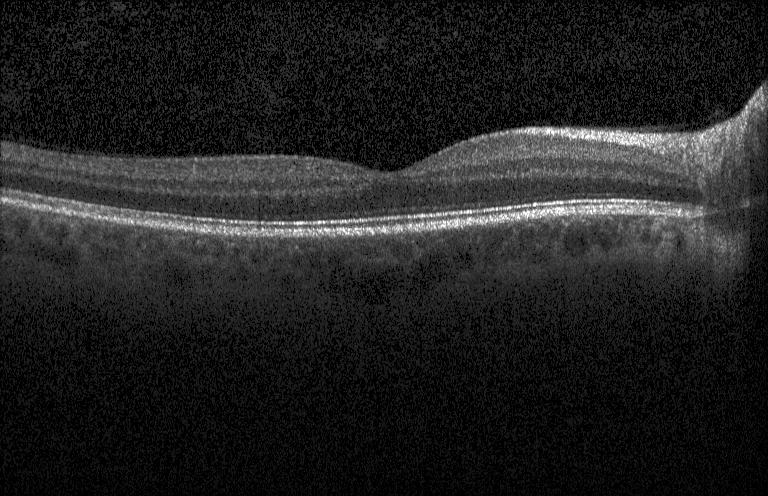

OCT finding: no choroidal neovascularization, no diabetic macular edema, and no drusen.